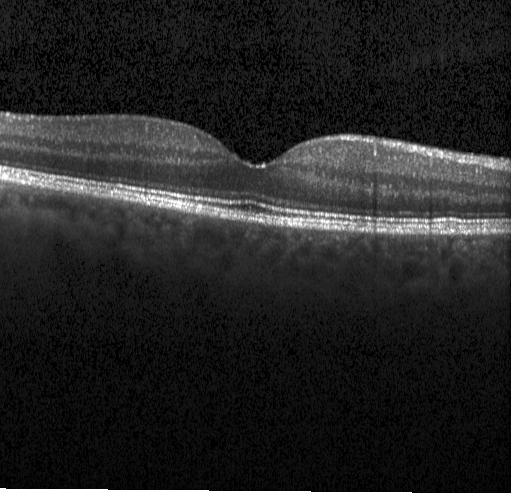
This B-scan demonstrates no evidence of CNV, DME, or drusen.